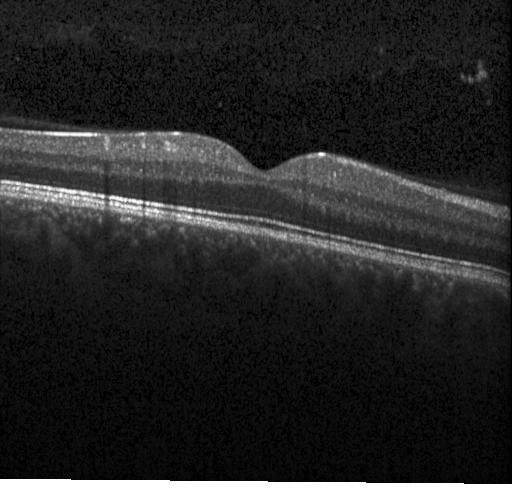 Spectral-domain optical coherence tomography; fovea-centered; OCT B-scan; Heidelberg Spectralis. Diagnosis: no evidence of choroidal neovascularization, diabetic macular edema, or drusen.